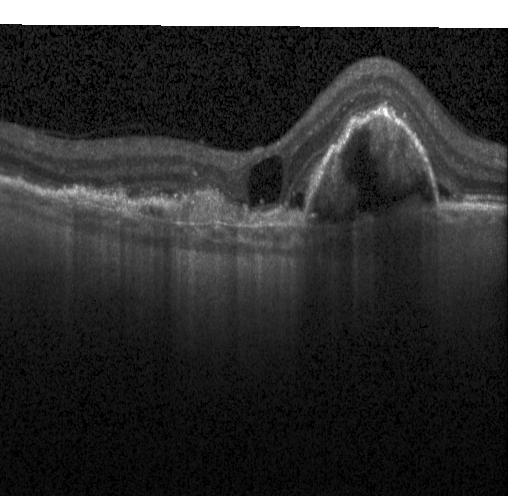

This B-scan demonstrates CNV.